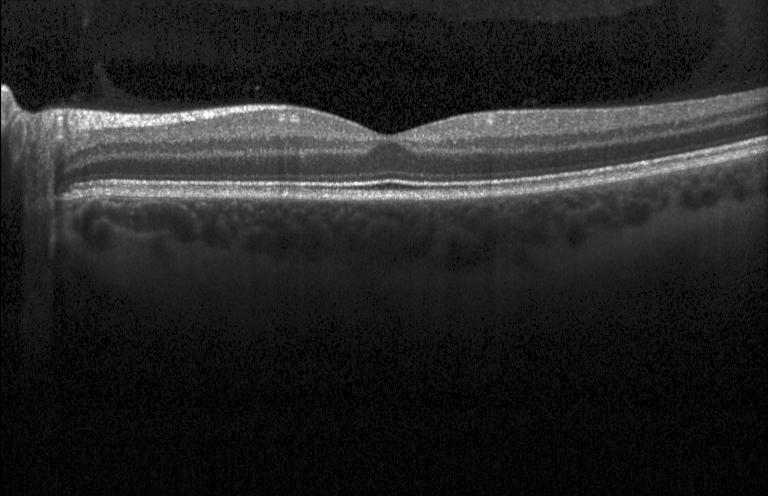

Dx: neither choroidal neovascularization, diabetic macular edema, nor drusen.